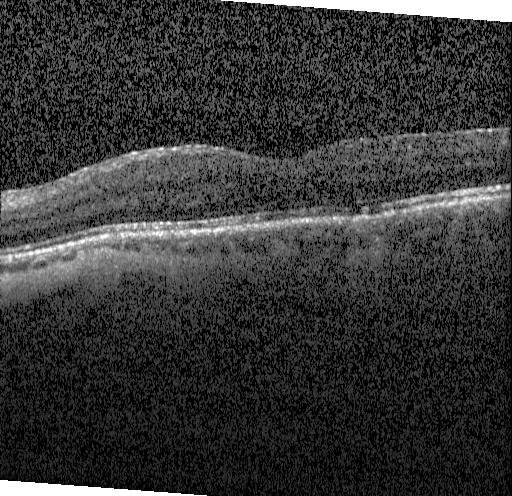
Finding: no choroidal neovascularization, diabetic macular edema, or drusen.